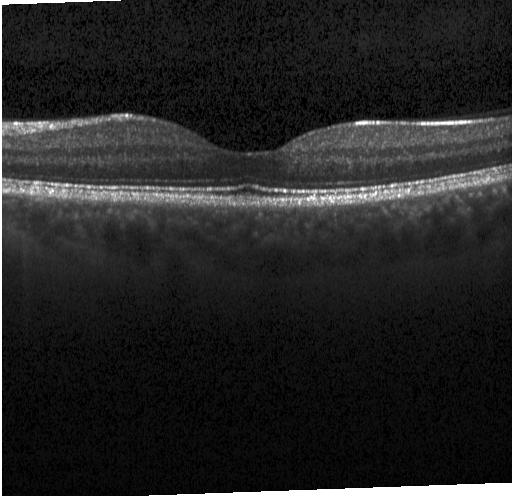 Spectral-domain OCT B-scan: neither choroidal neovascularization, diabetic macular edema, nor drusen.